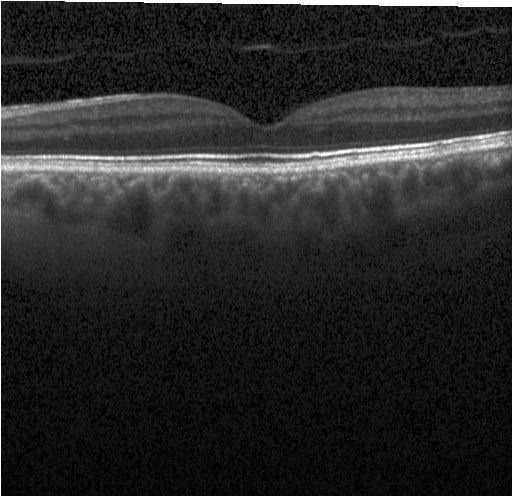
No choroidal neovascularization, diabetic macular edema, or drusen.